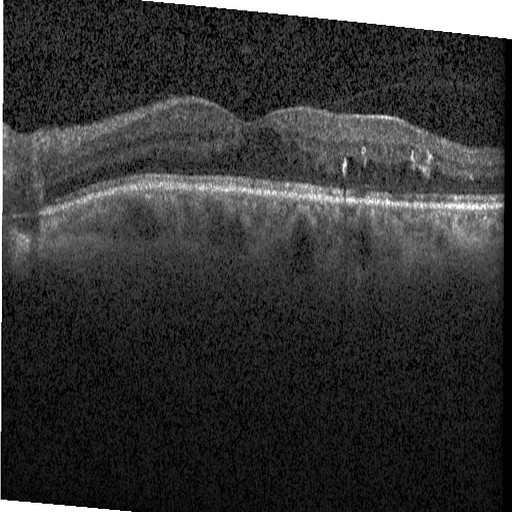
SD-OCT · centered on the fovea · Heidelberg Spectralis OCT system · OCT B-scan.
This B-scan demonstrates diabetic macular edema (DME).